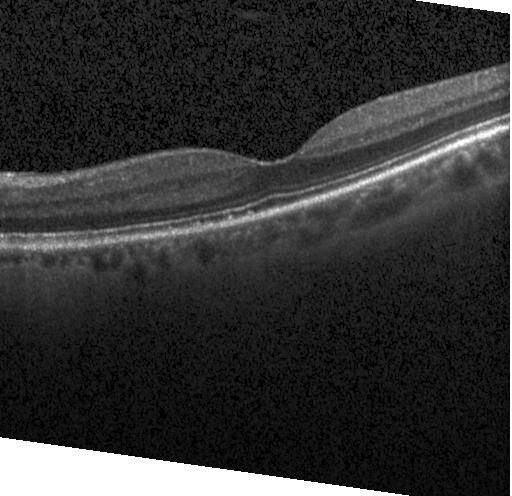 Retinal OCT B-scan — Macular OCT: no CNV, no DME, and no drusen.